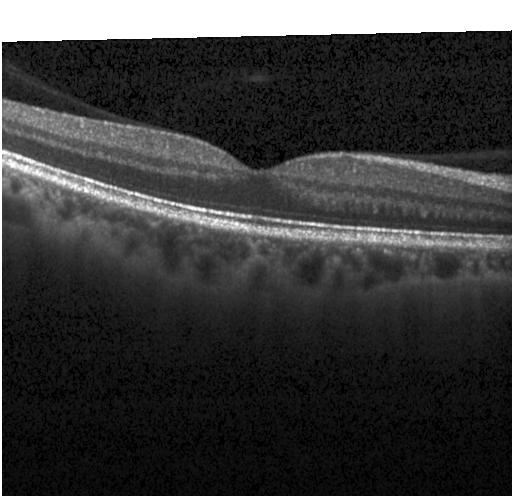

Centered on the fovea. Retinal OCT B-scan — Diagnosis: neither CNV, DME, nor drusen.